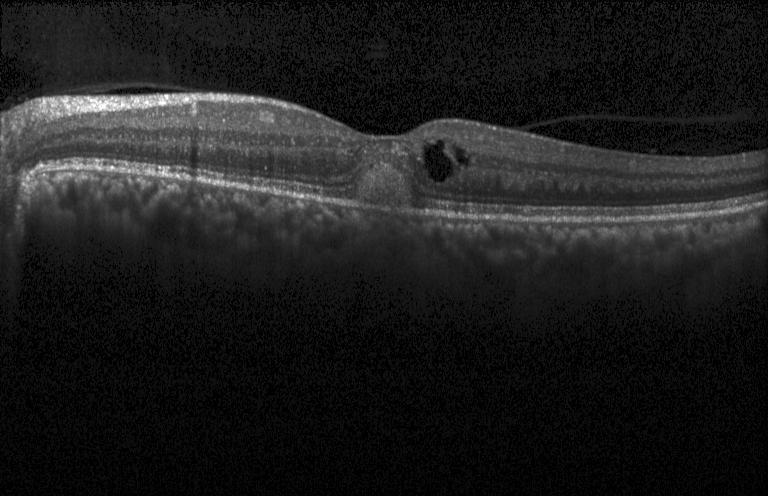
Spectral-domain OCT, macular scan, instrument: Heidelberg Spectralis, OCT B-scan
Macular OCT: CNV.